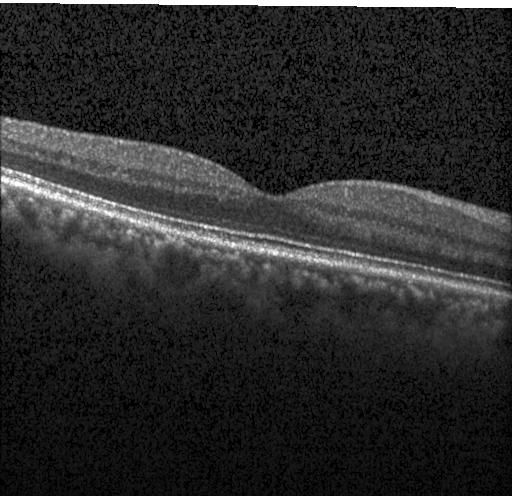 Diagnosis: no evidence of choroidal neovascularization, diabetic macular edema, or drusen.